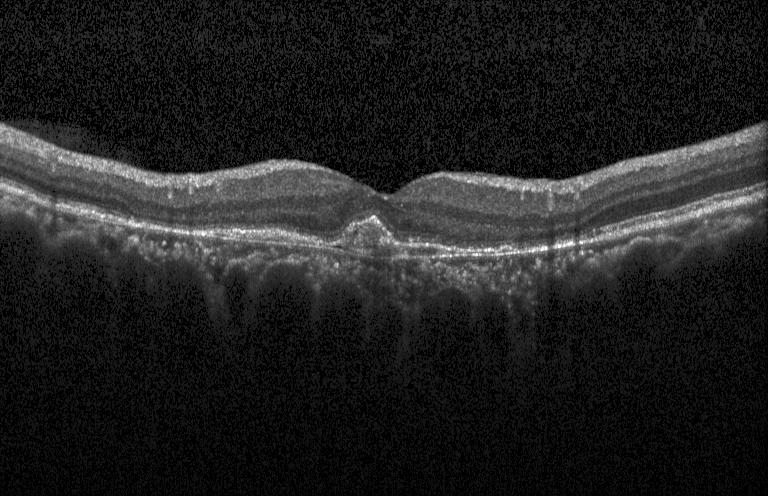

OCT line scan · through the macula. Impression: choroidal neovascularization (CNV).